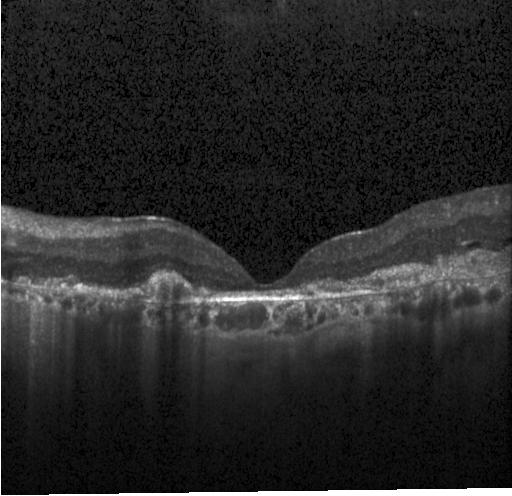
Macular OCT: choroidal neovascularization.